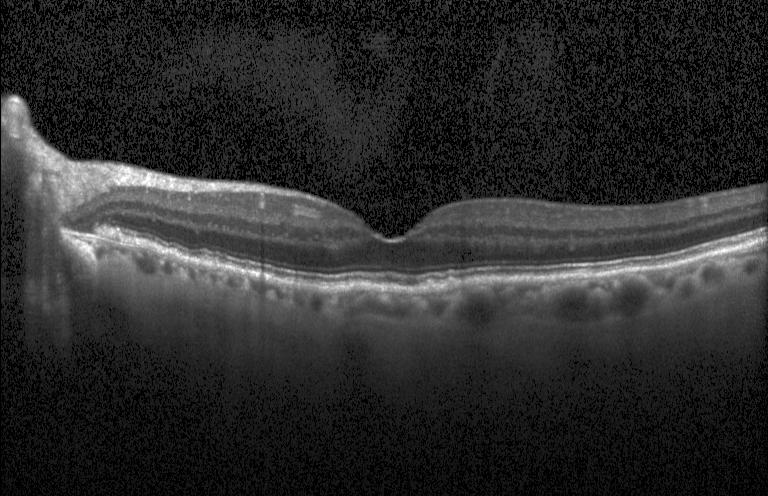
Optical coherence tomography scan · spectral-domain optical coherence tomography · macular scan.
Diagnosis: drusen.